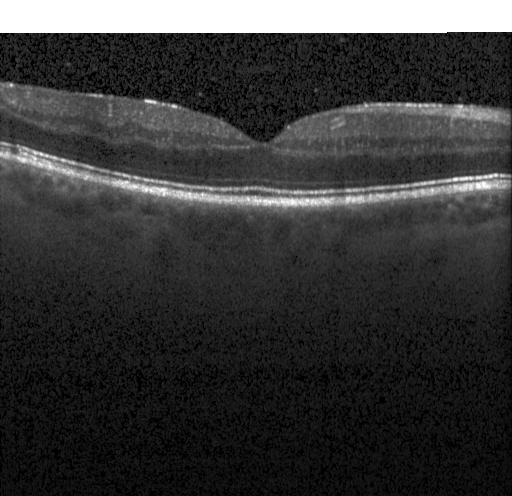
Horizontal scan through the fovea. SD-OCT. Optical coherence tomography B-scan. Heidelberg Spectralis.
Dx: neither choroidal neovascularization, diabetic macular edema, nor drusen.